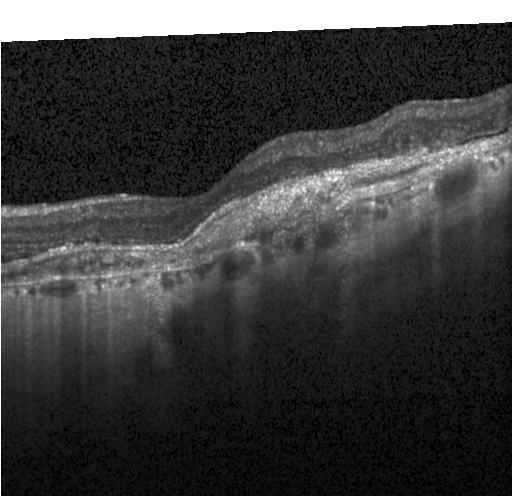

Optical coherence tomography scan.
Finding: choroidal neovascularization (CNV).